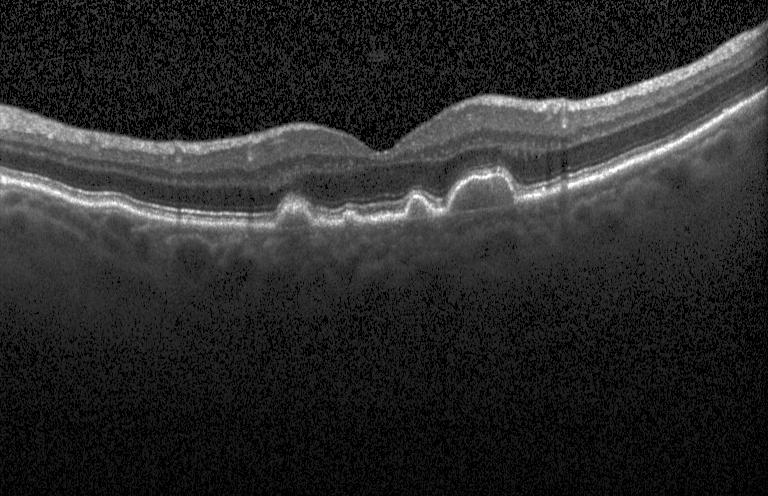
Assessment: drusen.